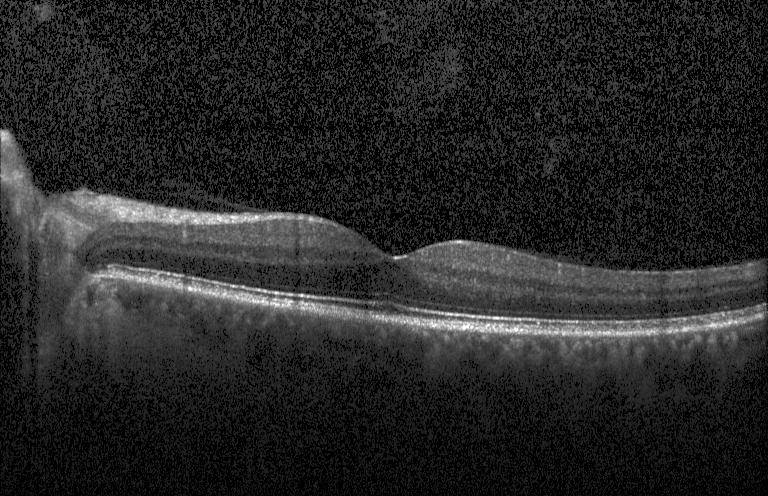
Finding: neither choroidal neovascularization, diabetic macular edema, nor drusen.